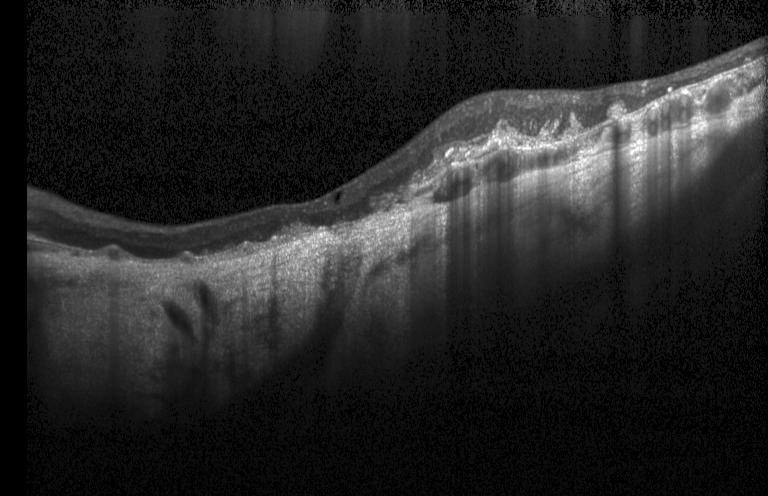

OCT line scan — Diagnosis: choroidal neovascularization (CNV).